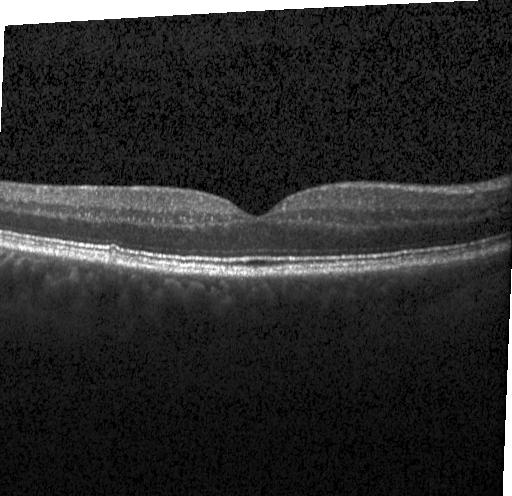

Diagnosis: neither choroidal neovascularization, diabetic macular edema, nor drusen.